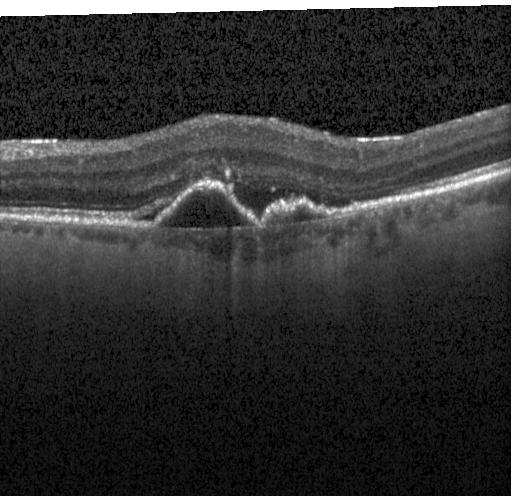

Horizontal scan through the fovea; spectral-domain OCT; Heidelberg Spectralis; OCT B-scan — Impression: choroidal neovascularization.